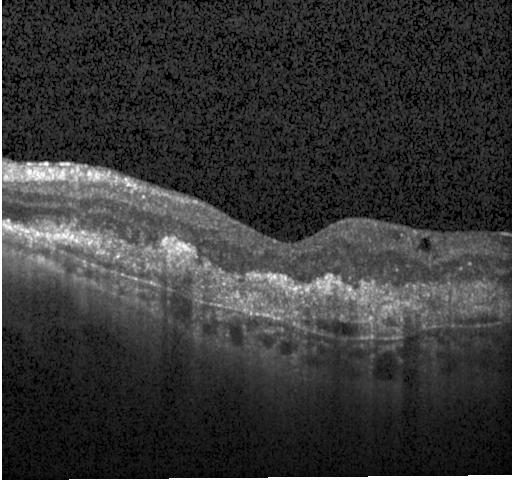 Spectral-domain optical coherence tomography. Heidelberg Spectralis. Macular scan. OCT line scan
Impression: a choroidal neovascular membrane.